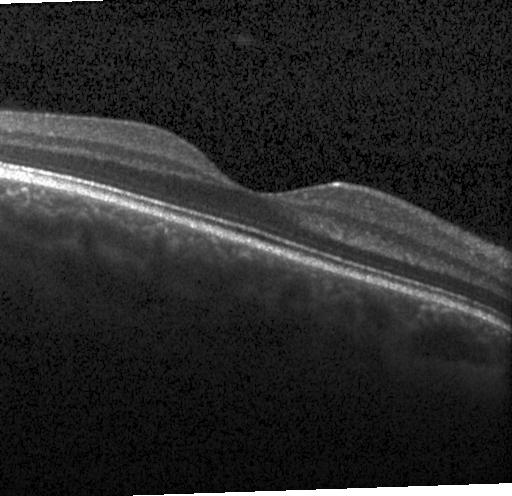 OCT line scan. Acquired on a Heidelberg Spectralis — Diagnosis: neither choroidal neovascularization, diabetic macular edema, nor drusen.